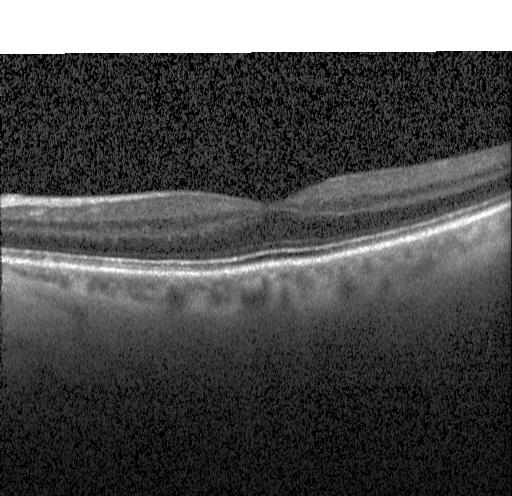

Diagnosis: no CNV, DME, or drusen.